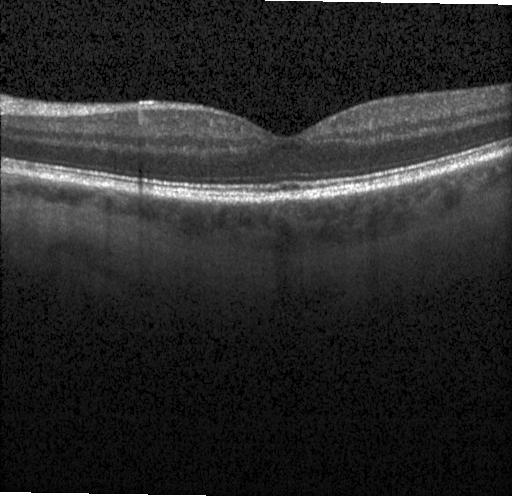

Acquired on a Heidelberg Spectralis. Spectral-domain optical coherence tomography. Fovea-centered. OCT B-scan. Finding: no choroidal neovascularization, diabetic macular edema, or drusen.